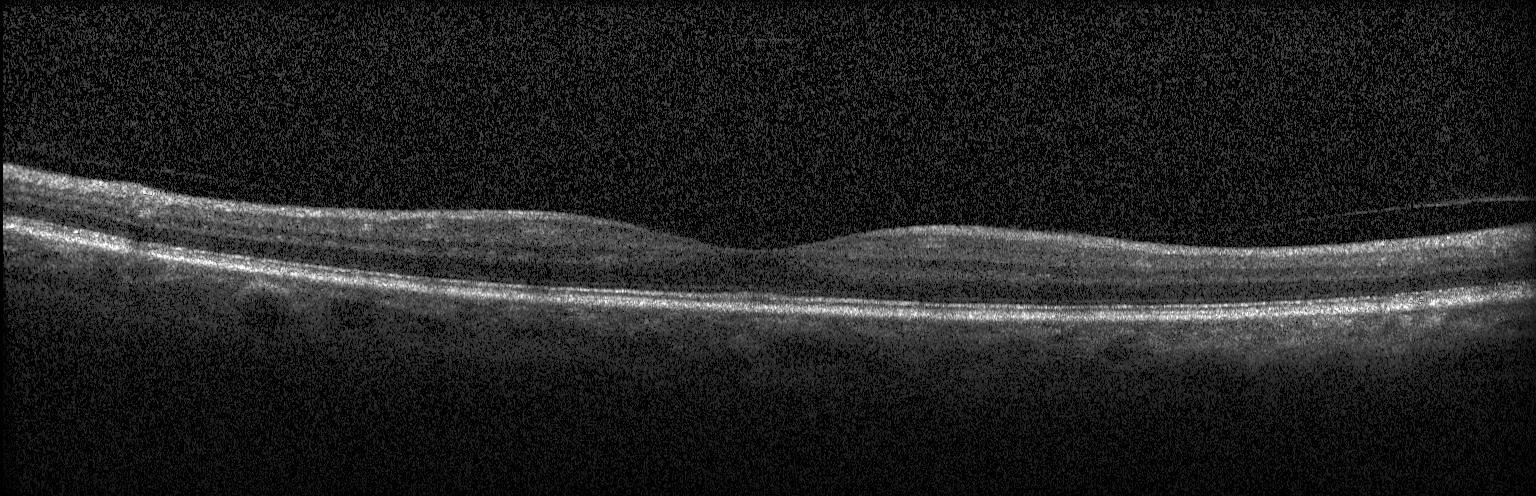
OCT finding: no CNV, DME, or drusen.